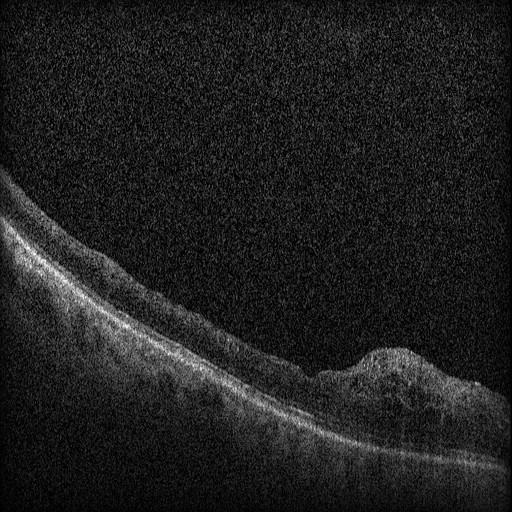 Horizontal scan through the fovea, SD-OCT, optical coherence tomography scan — Finding: DME.